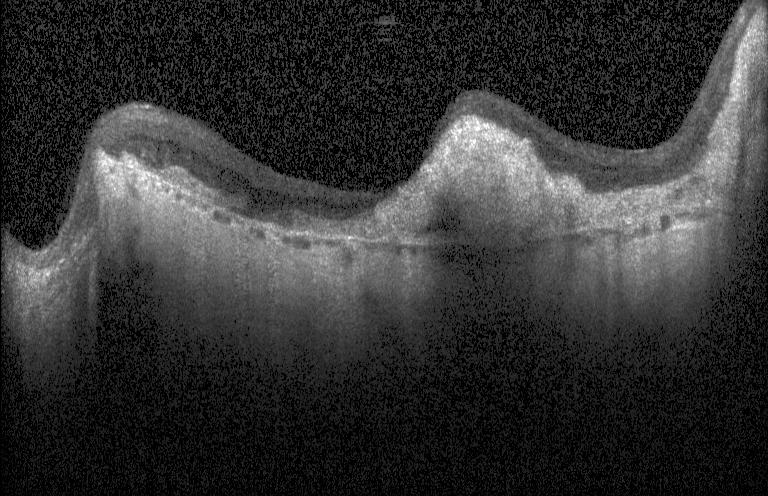
OCT finding: choroidal neovascularization (CNV).